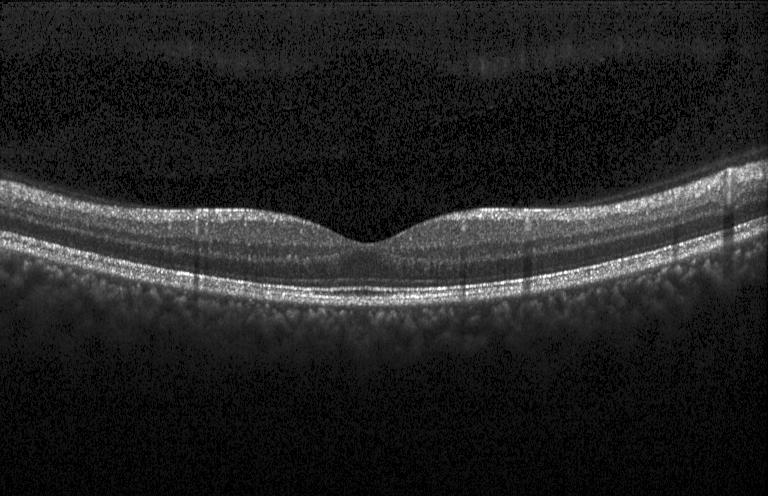
Instrument: Heidelberg Spectralis, optical coherence tomography scan, spectral-domain OCT — Diagnosis: no CNV, no DME, and no drusen.